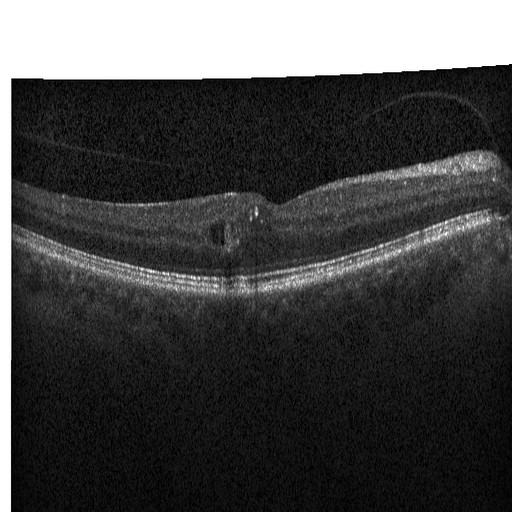
The scan shows diabetic macular edema (DME).